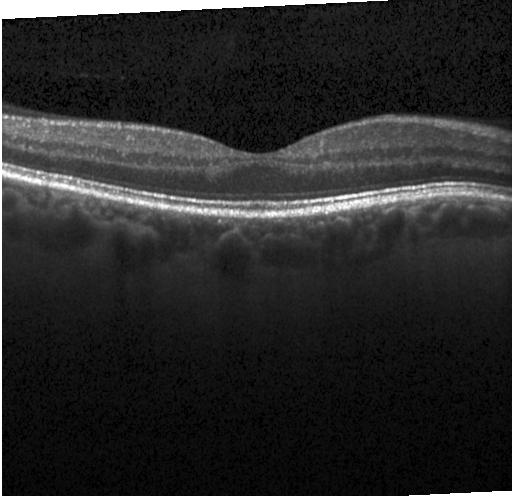

Instrument: Heidelberg Spectralis. Retinal OCT B-scan. Macular scan. SD-OCT
The scan shows no choroidal neovascularization, no diabetic macular edema, and no drusen.